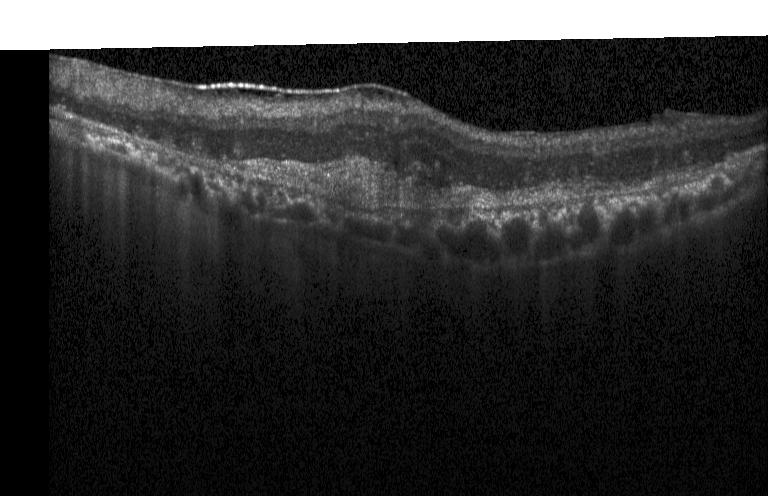 Optical coherence tomography B-scan. Impression: a choroidal neovascular membrane.